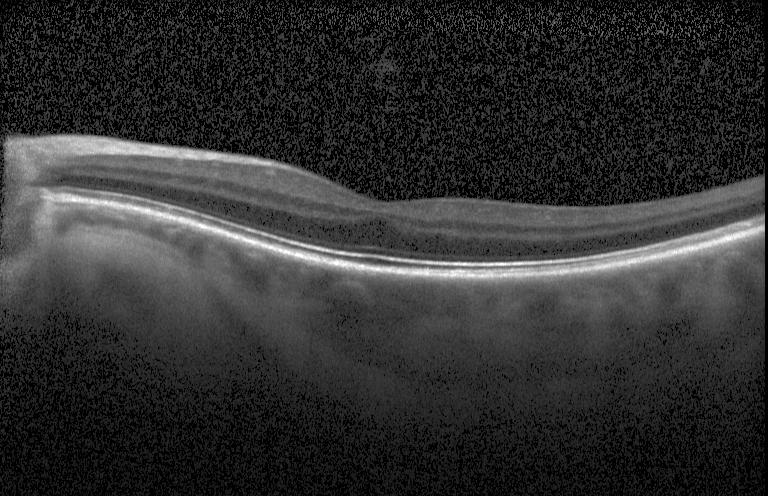
Finding: no choroidal neovascularization, no diabetic macular edema, and no drusen.